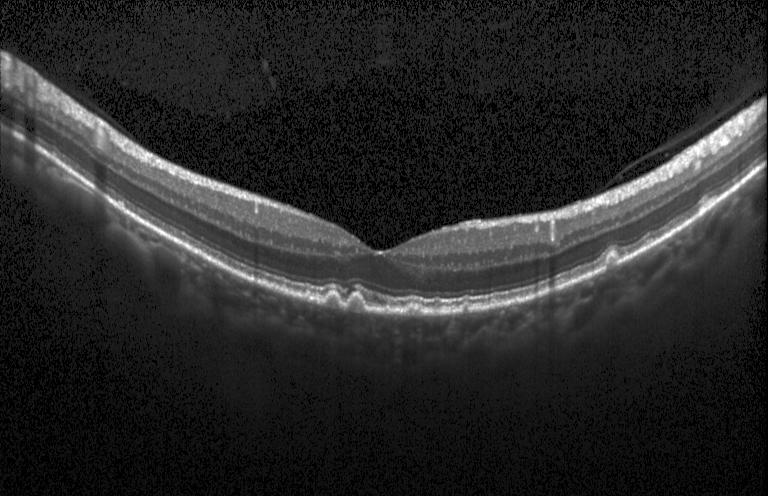 Optical coherence tomography B-scan; acquired on a Heidelberg Spectralis; horizontal scan through the fovea.
Assessment: drusen.